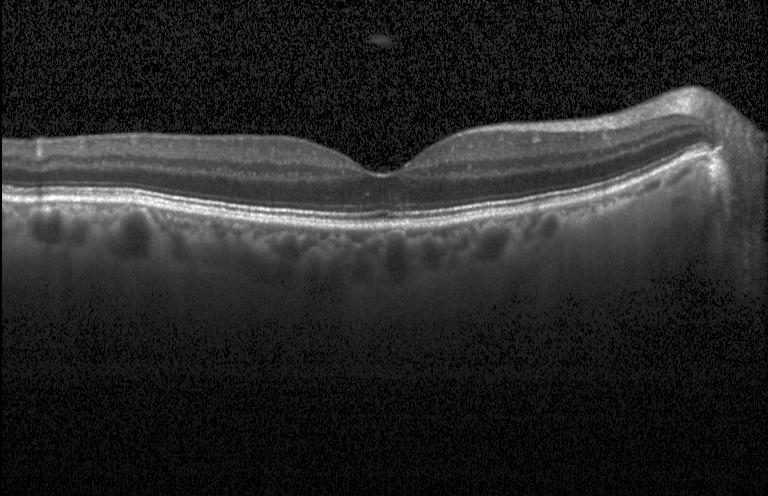
Acquired on a Heidelberg Spectralis, OCT B-scan — Assessment: no CNV, no DME, and no drusen.